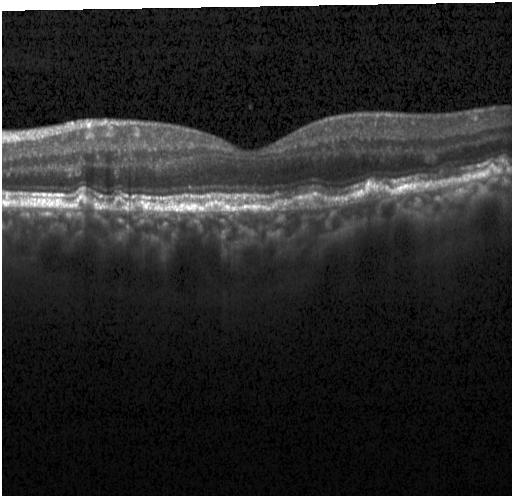

Impression: drusen.